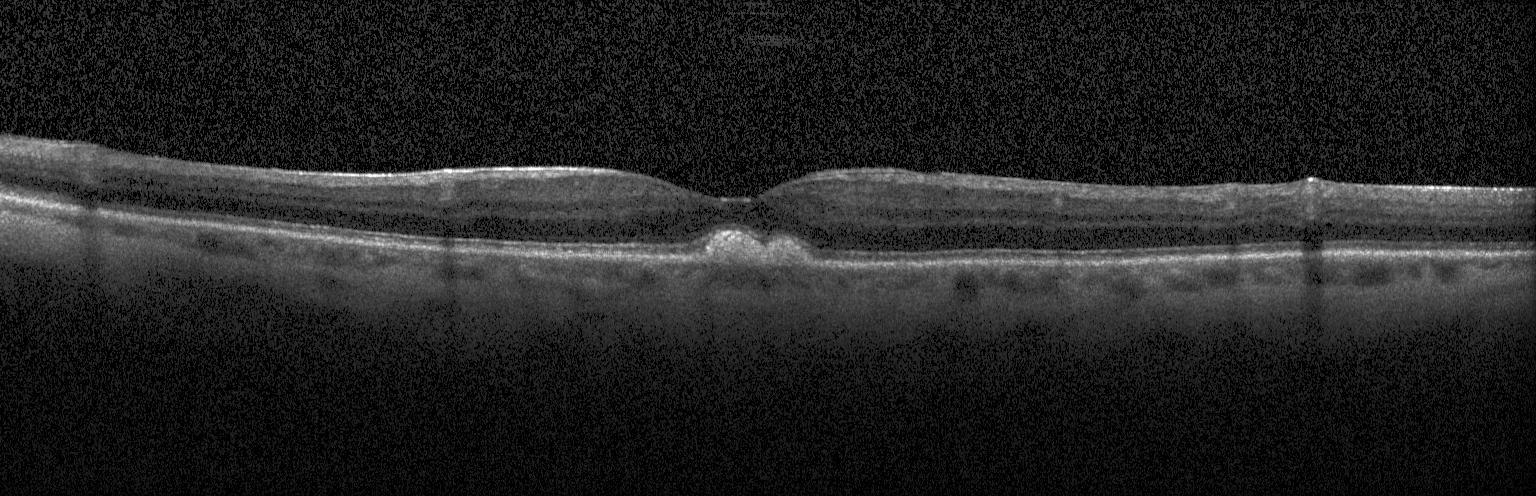
Finding: drusen.